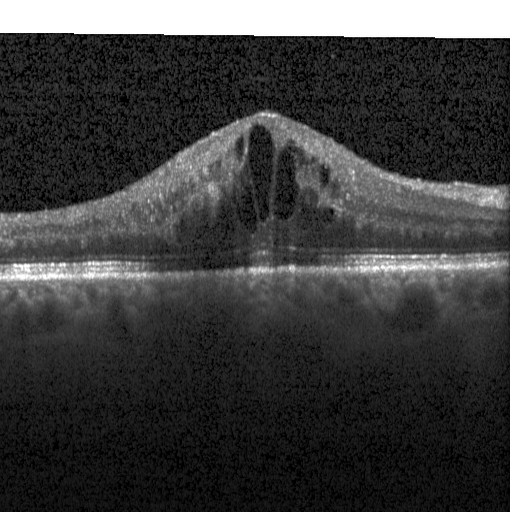
Diagnosis: diabetic macular edema.